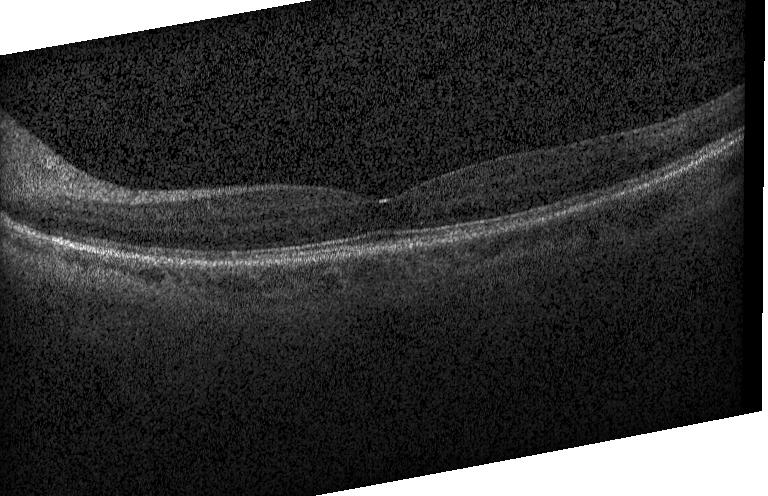 Optical coherence tomography B-scan; instrument: Heidelberg Spectralis; spectral-domain optical coherence tomography — Dx: neither CNV, DME, nor drusen.